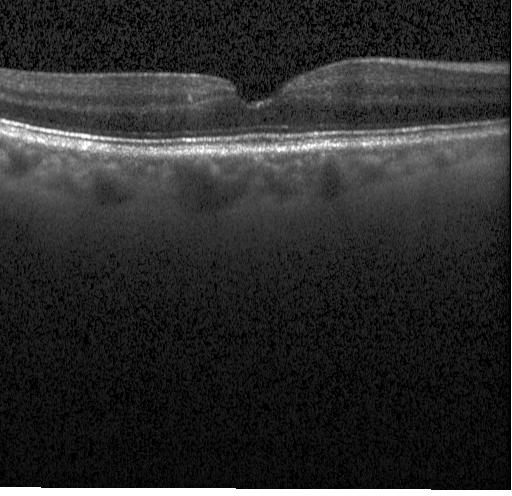

Finding: no choroidal neovascularization, diabetic macular edema, or drusen.